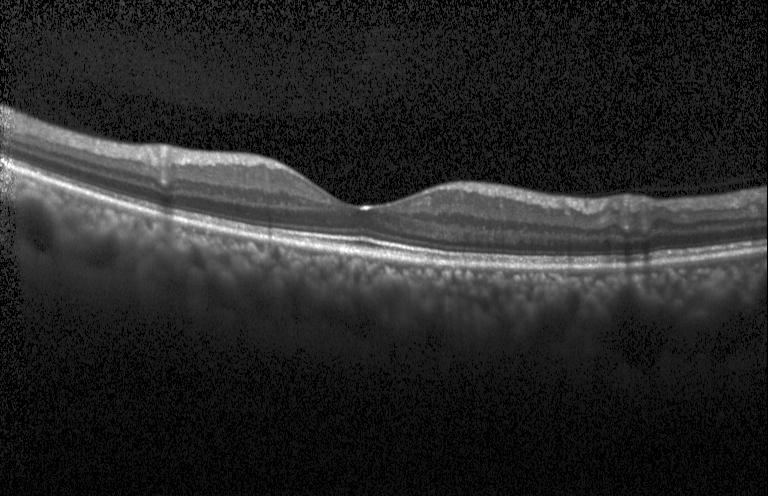 Finding: no choroidal neovascularization, no diabetic macular edema, and no drusen.